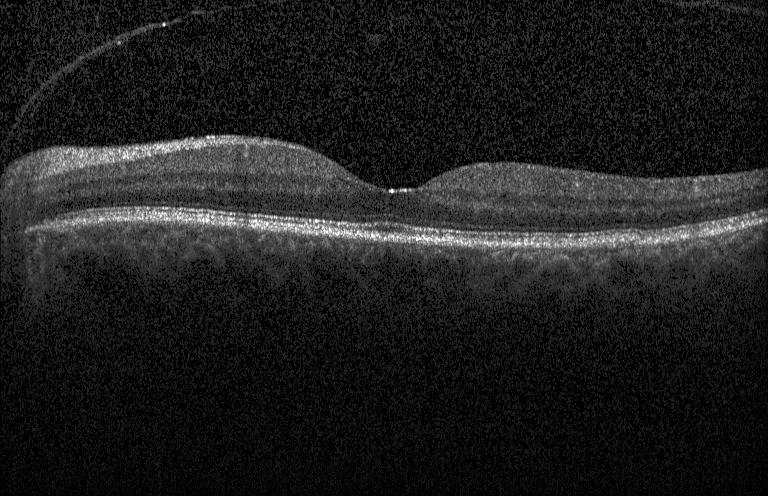 OCT finding: no evidence of CNV, DME, or drusen.